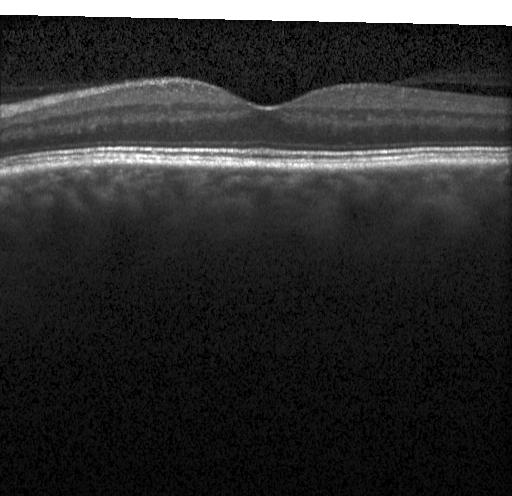
The scan shows no choroidal neovascularization, diabetic macular edema, or drusen.